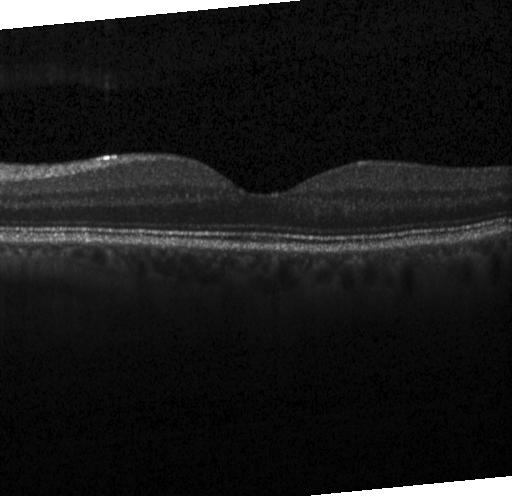
Instrument: Heidelberg Spectralis, centered on the fovea, OCT line scan.
Assessment: neither choroidal neovascularization, diabetic macular edema, nor drusen.